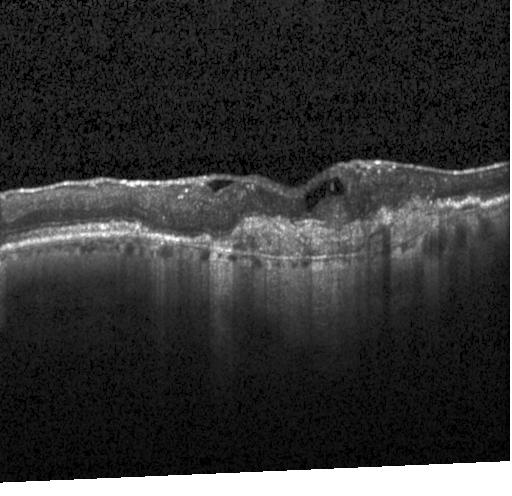
Retinal OCT cross-section showing a choroidal neovascular membrane.